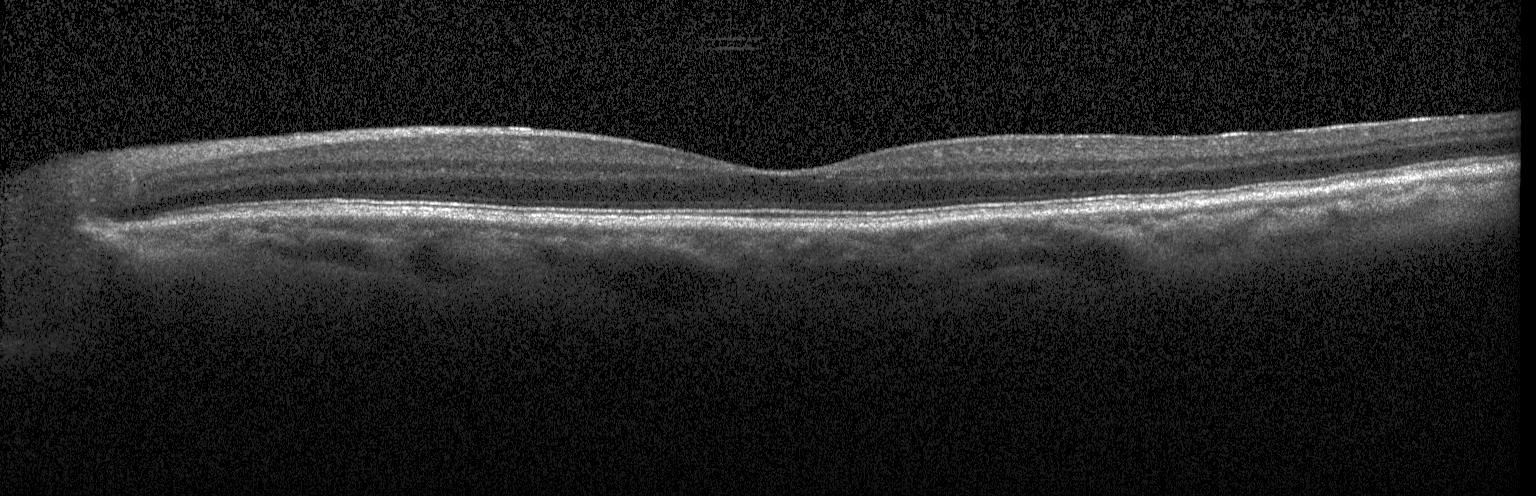
Instrument: Heidelberg Spectralis; centered on the fovea; retinal OCT B-scan; SD-OCT.
Diagnosis: no evidence of choroidal neovascularization, diabetic macular edema, or drusen.